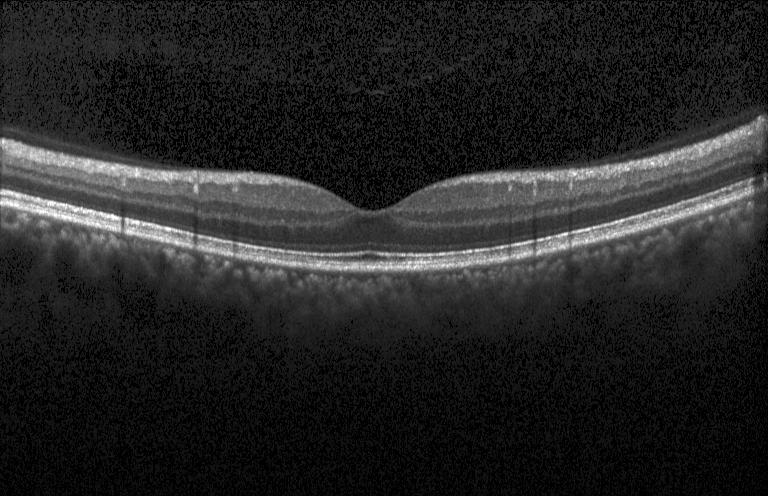 Optical coherence tomography scan. SD-OCT. Heidelberg Spectralis. Macular scan
The scan shows no choroidal neovascularization, diabetic macular edema, or drusen.